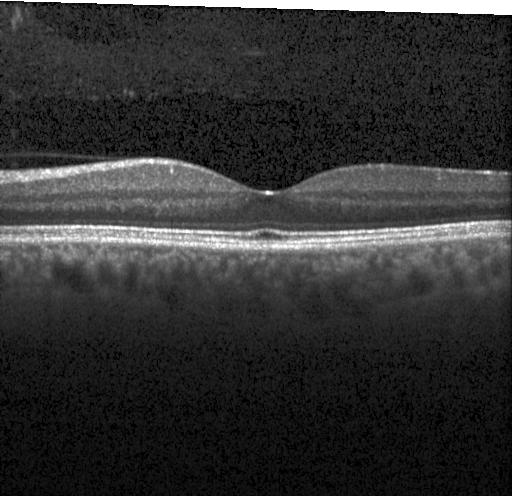
OCT scan showing no evidence of choroidal neovascularization, diabetic macular edema, or drusen.